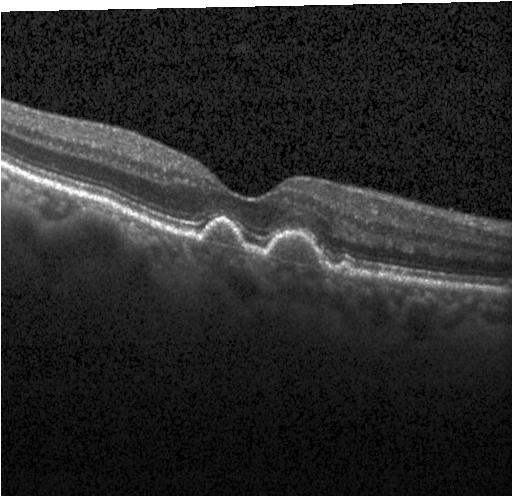 Optical coherence tomography scan. Impression: multiple drusen.